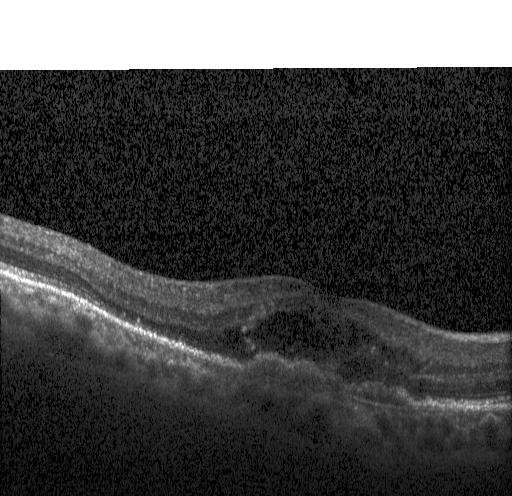 Macular OCT: choroidal neovascularization.